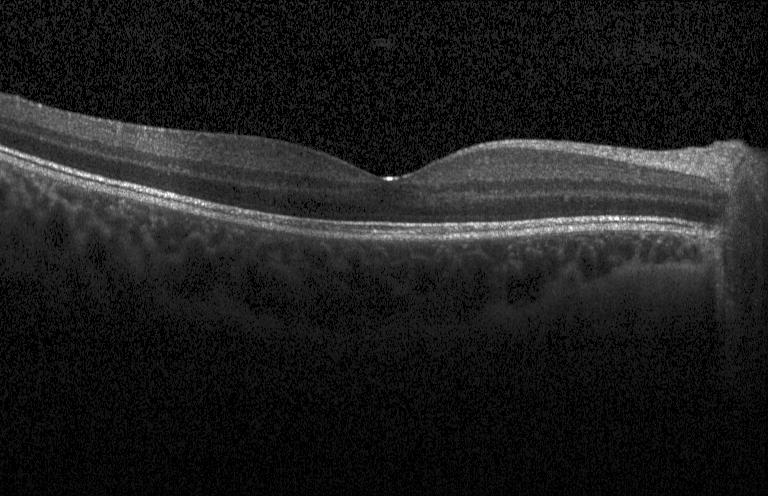
OCT line scan.
Diagnosis: neither choroidal neovascularization, diabetic macular edema, nor drusen.